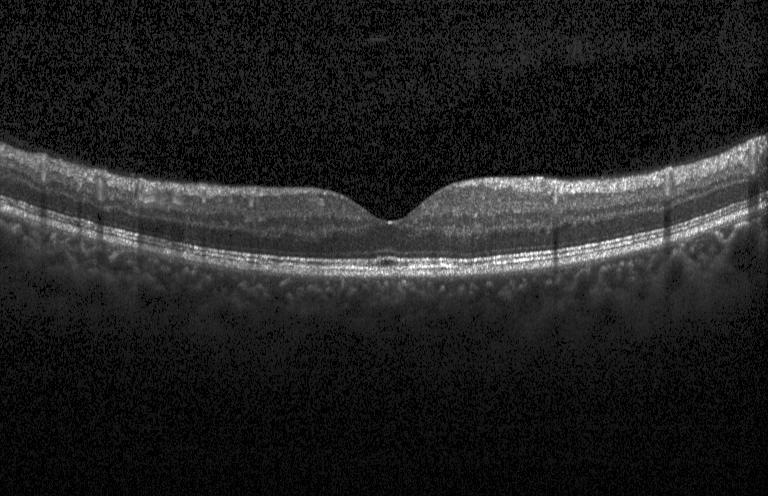

Retinal OCT cross-section. Heidelberg Spectralis OCT system — Dx: no evidence of choroidal neovascularization, diabetic macular edema, or drusen.